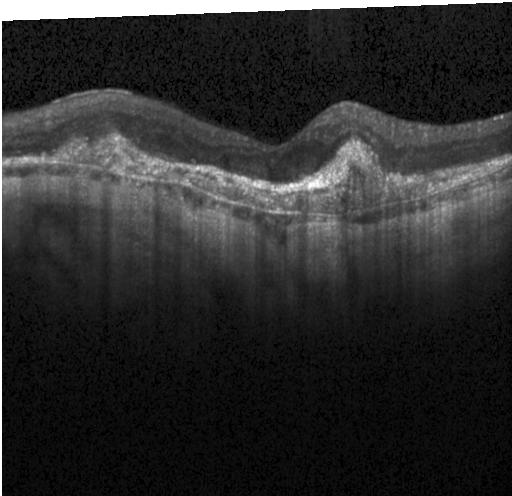

Finding: a choroidal neovascular membrane.